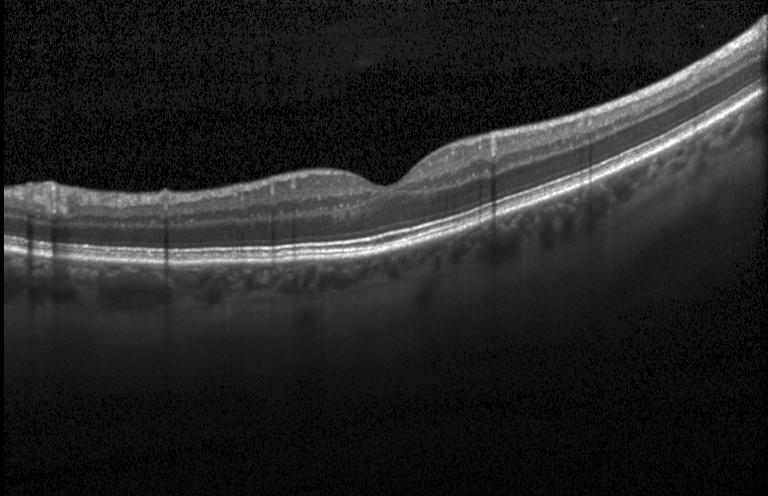

Macular OCT: no evidence of CNV, DME, or drusen.